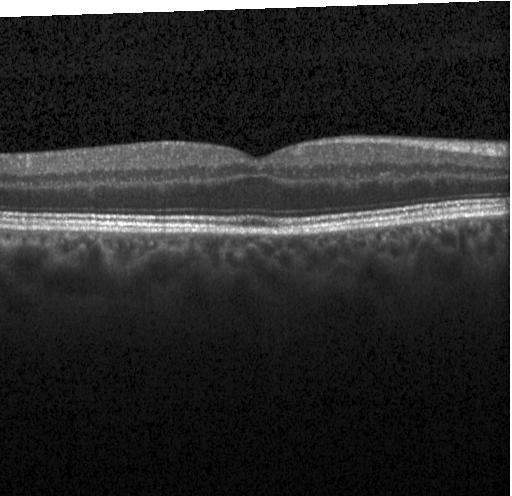 Diagnosis: neither choroidal neovascularization, diabetic macular edema, nor drusen.